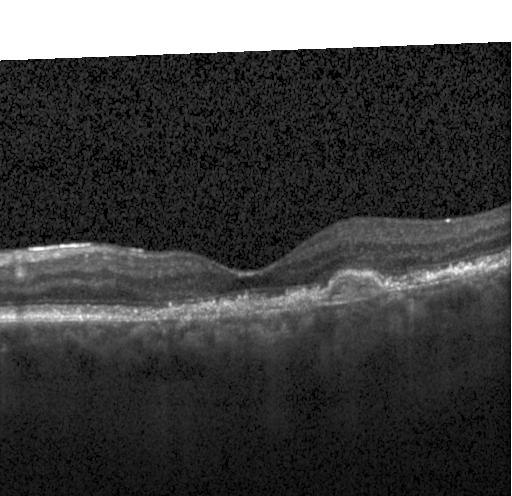
Impression: a choroidal neovascular membrane.